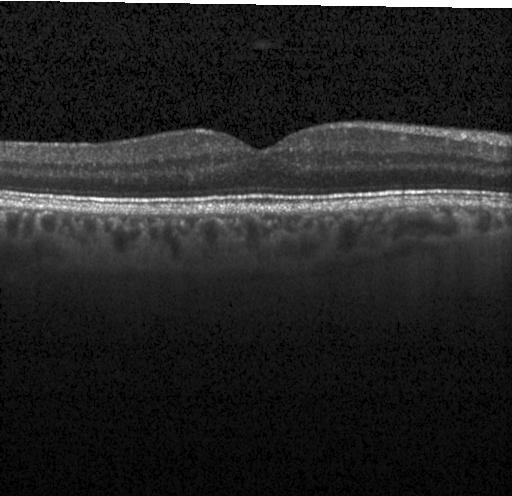

Instrument: Heidelberg Spectralis, OCT B-scan, centered on the fovea.
OCT finding: neither choroidal neovascularization, diabetic macular edema, nor drusen.